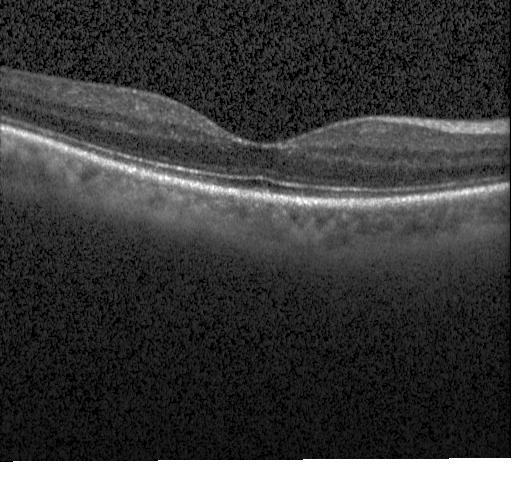 Macular scan; OCT B-scan — Finding: no CNV, DME, or drusen.